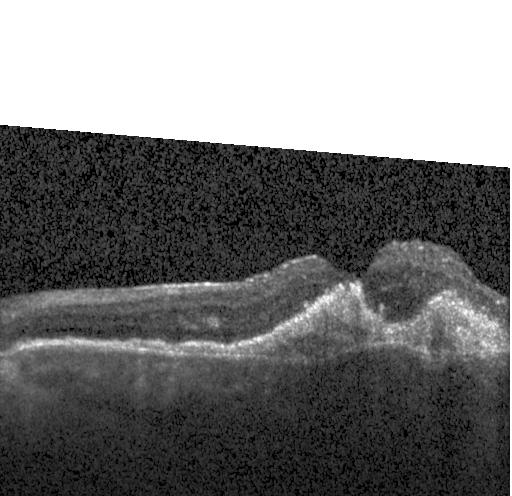

Heidelberg Spectralis OCT system; horizontal scan through the fovea; OCT line scan; spectral-domain OCT. Dx: choroidal neovascularization (CNV).